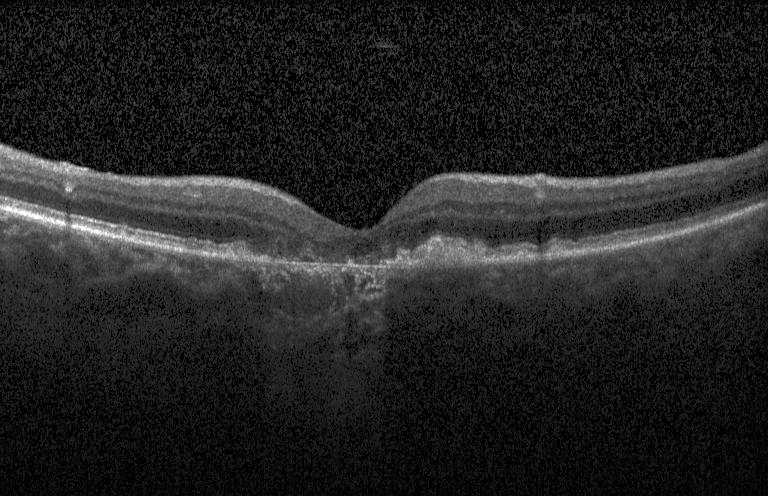 Spectral-domain OCT, Heidelberg Spectralis OCT system, retinal OCT B-scan
Assessment: a choroidal neovascular membrane.